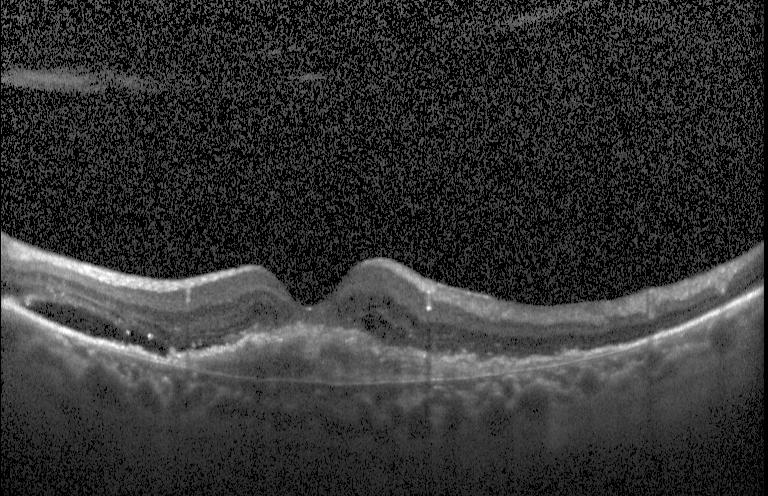 Spectral-domain OCT B-scan: a choroidal neovascular membrane.